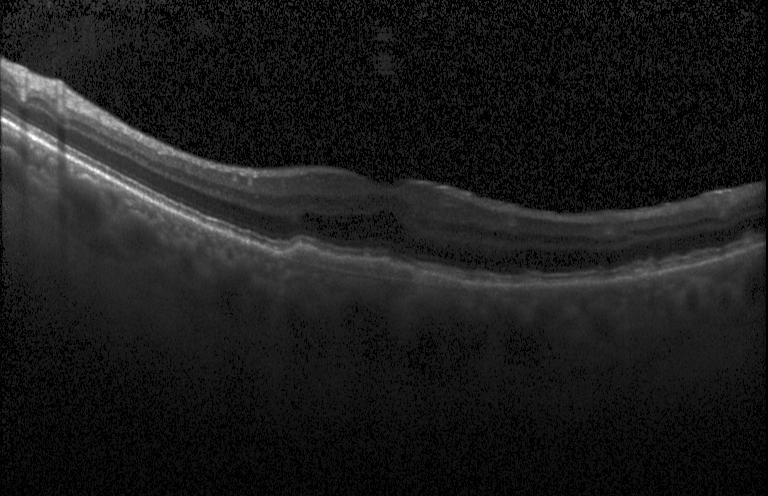
Retinal OCT B-scan. This B-scan demonstrates CNV.